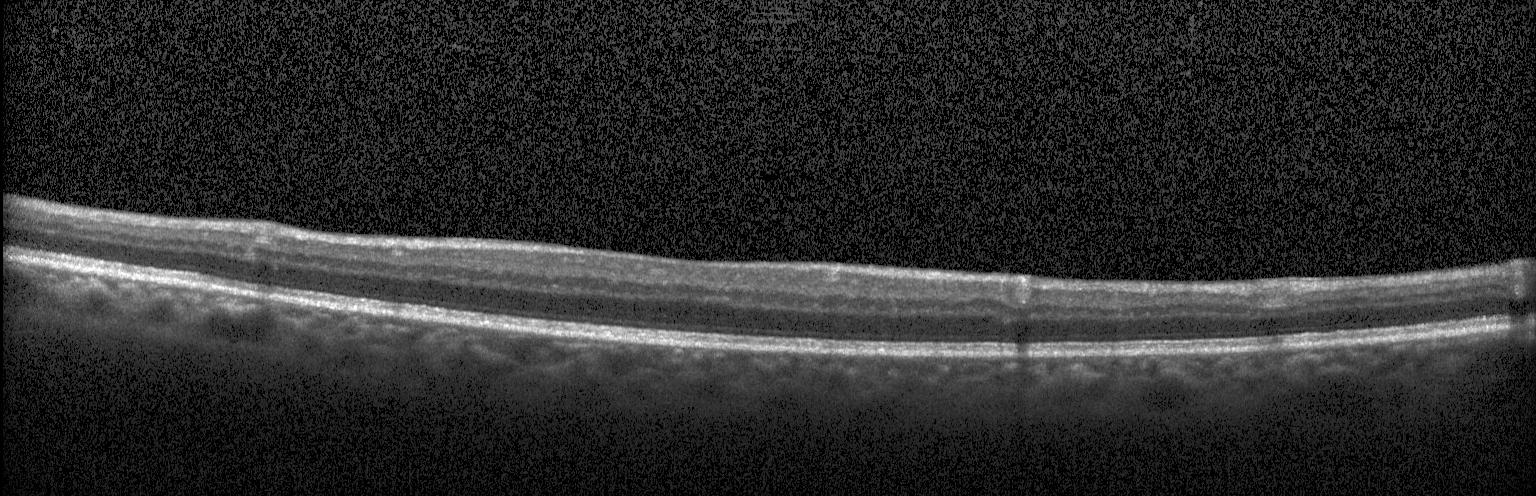
Instrument: Heidelberg Spectralis · fovea-centered · optical coherence tomography scan · spectral-domain OCT.
The scan shows neither choroidal neovascularization, diabetic macular edema, nor drusen.